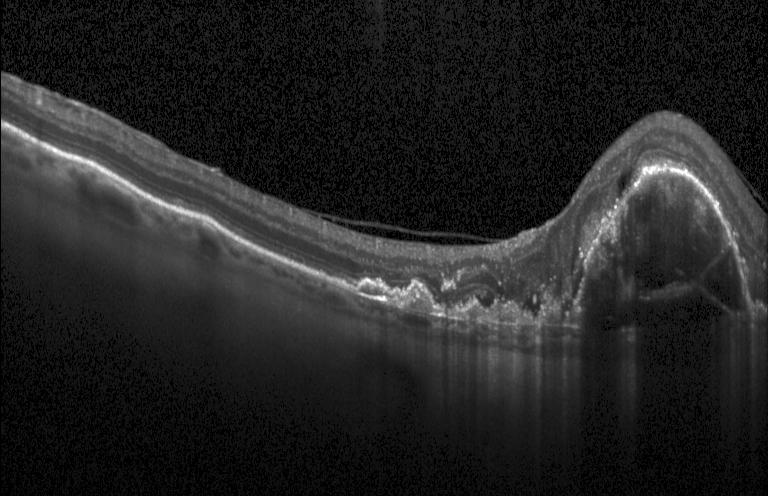

OCT B-scan · Heidelberg Spectralis · macular scan
Impression: a choroidal neovascular membrane.